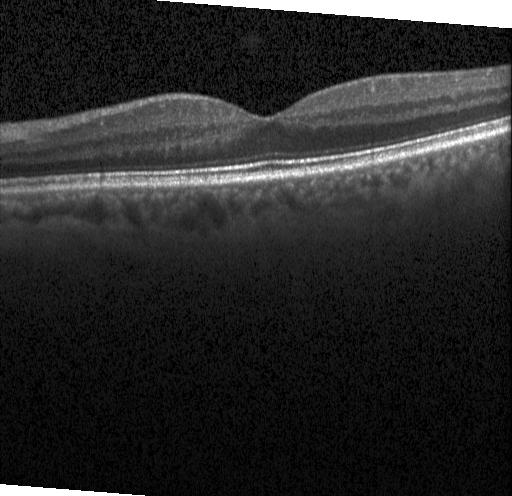

Retinal OCT cross-section; through the macula; spectral-domain optical coherence tomography — Impression: no evidence of choroidal neovascularization, diabetic macular edema, or drusen.